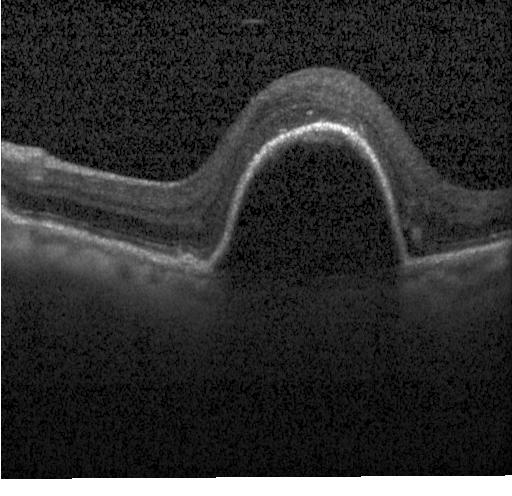
Macular OCT: a choroidal neovascular membrane.